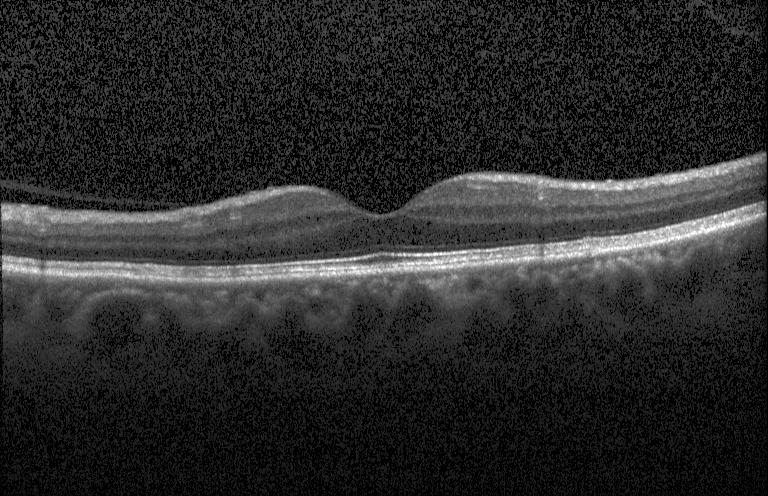

Optical coherence tomography scan · acquired on a Heidelberg Spectralis · centered on the fovea · SD-OCT — Finding: no evidence of choroidal neovascularization, diabetic macular edema, or drusen.